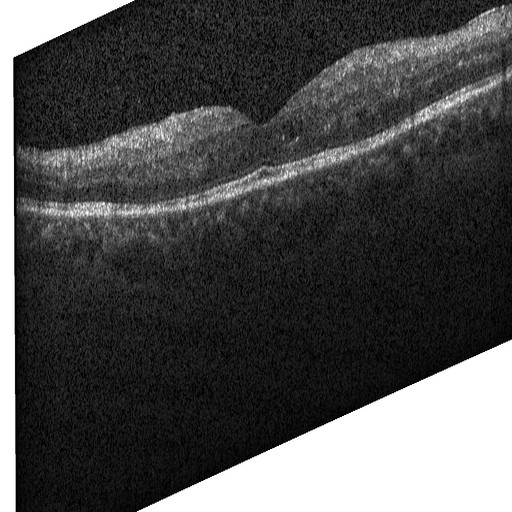
Acquired on a Heidelberg Spectralis, SD-OCT, retinal OCT B-scan. The scan shows DME.